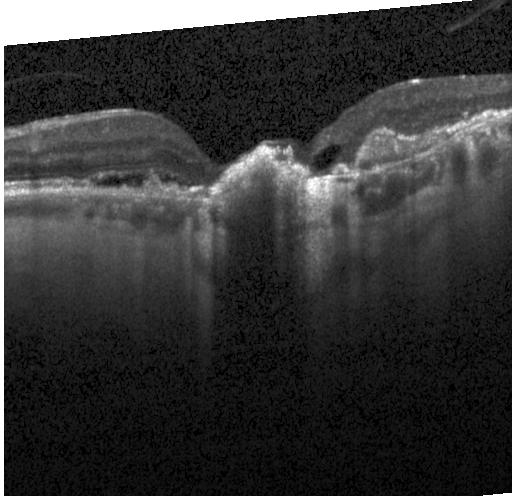

Dx: choroidal neovascularization (CNV).